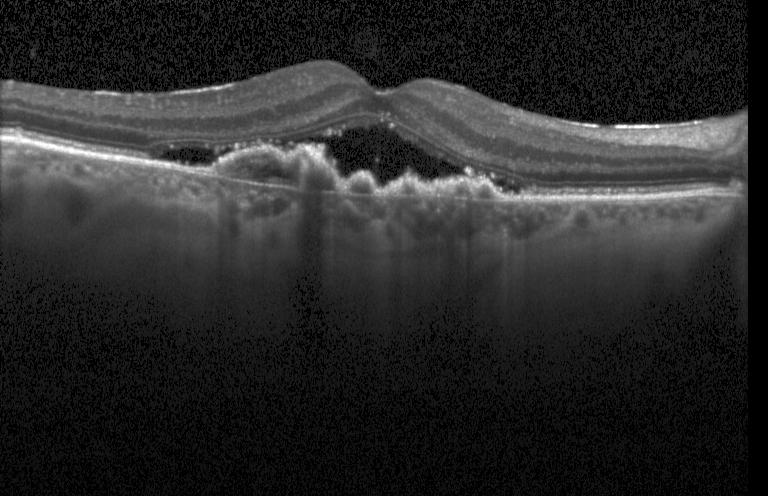
A choroidal neovascular membrane.